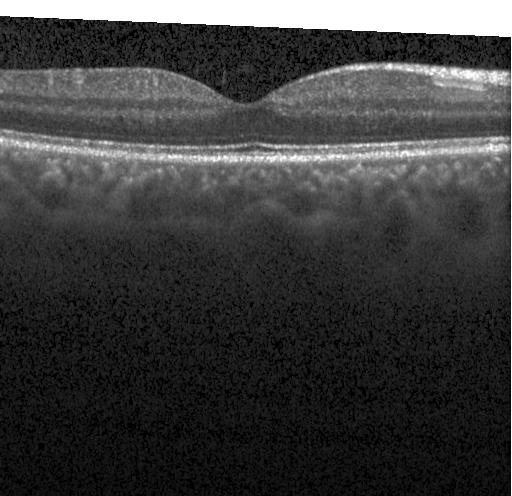
Diagnosis: no evidence of CNV, DME, or drusen.